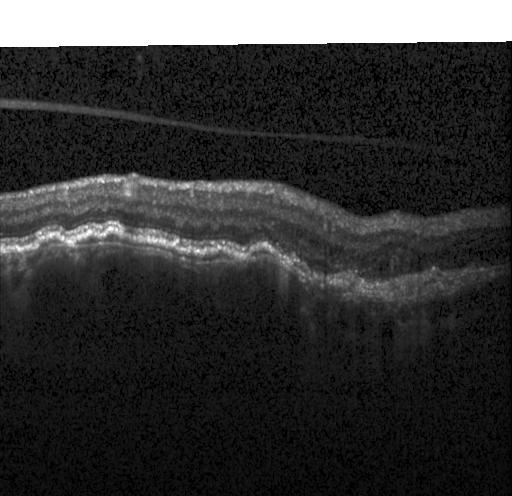 OCT B-scan. Diagnosis: a choroidal neovascular membrane.